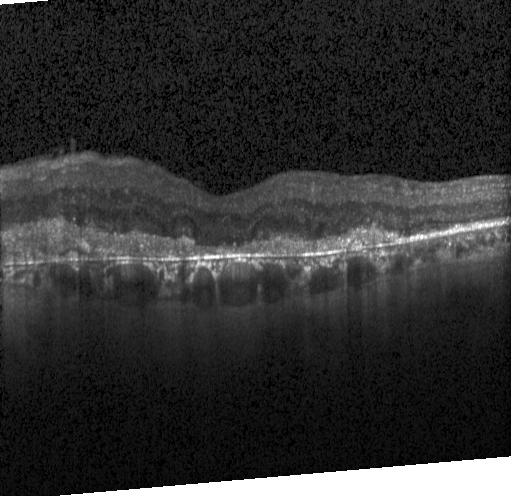 OCT finding: a choroidal neovascular membrane.